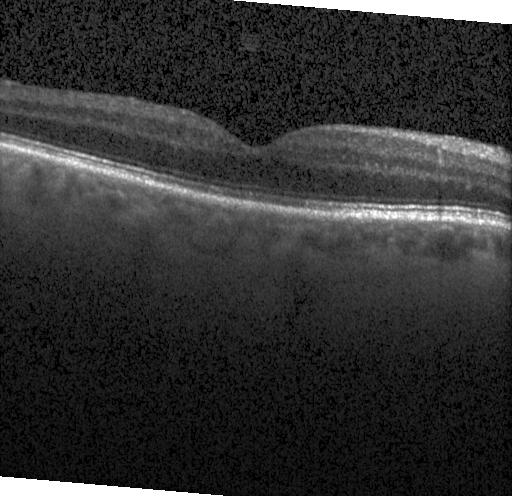
Retinal OCT cross-section; spectral-domain OCT. Macular OCT: no choroidal neovascularization, no diabetic macular edema, and no drusen.